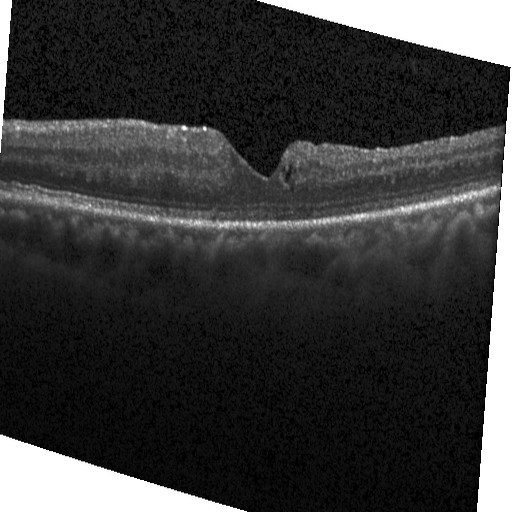
Instrument: Heidelberg Spectralis · centered on the fovea · spectral-domain optical coherence tomography · optical coherence tomography B-scan. Impression: DME.